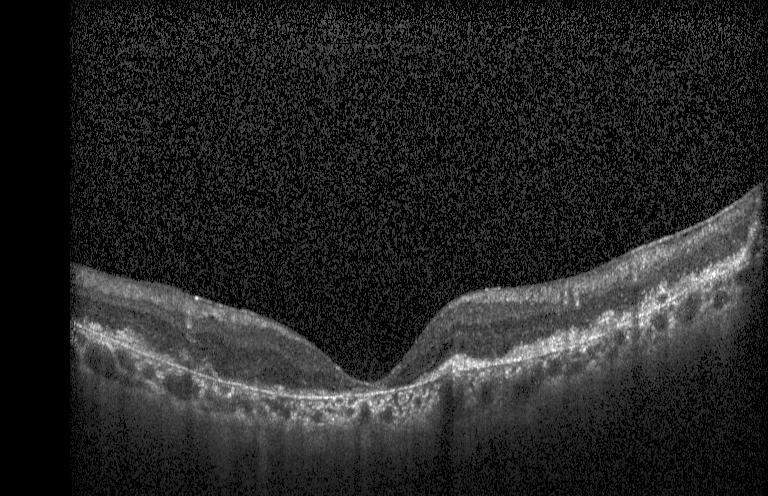 Optical coherence tomography scan — Finding: choroidal neovascularization (CNV).